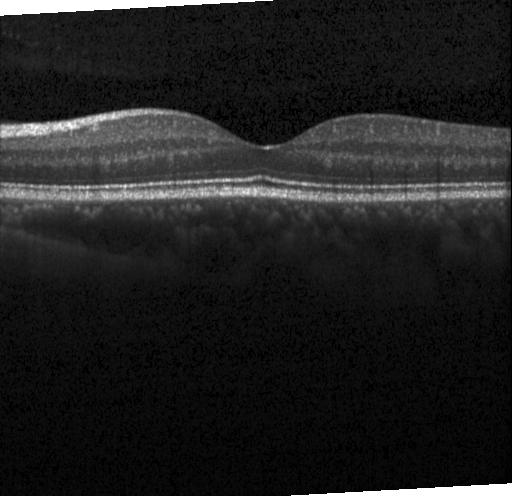 Optical coherence tomography scan; macular scan; Heidelberg Spectralis OCT system
Impression: no evidence of choroidal neovascularization, diabetic macular edema, or drusen.